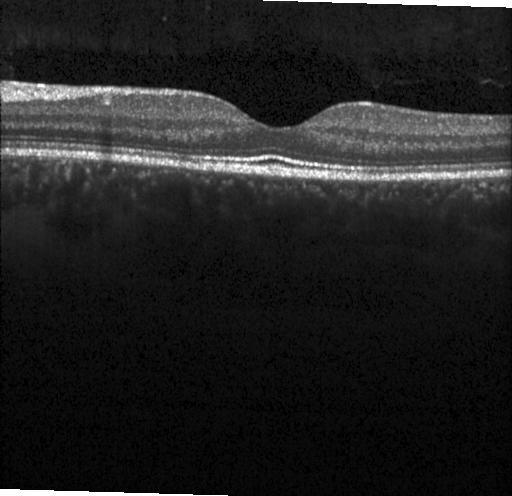

Horizontal scan through the fovea, OCT B-scan, Heidelberg Spectralis, SD-OCT — Macular OCT: no choroidal neovascularization, diabetic macular edema, or drusen.